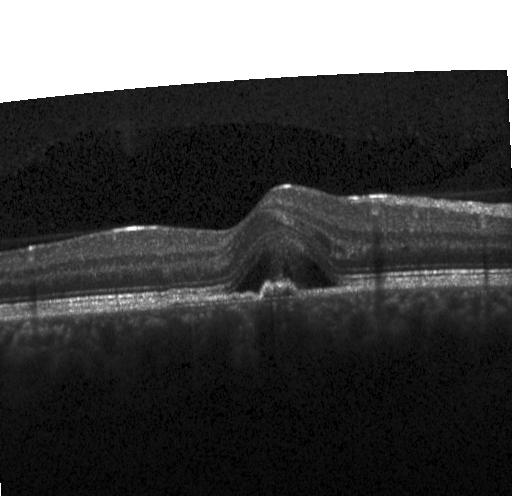

OCT B-scan. Impression: CNV.